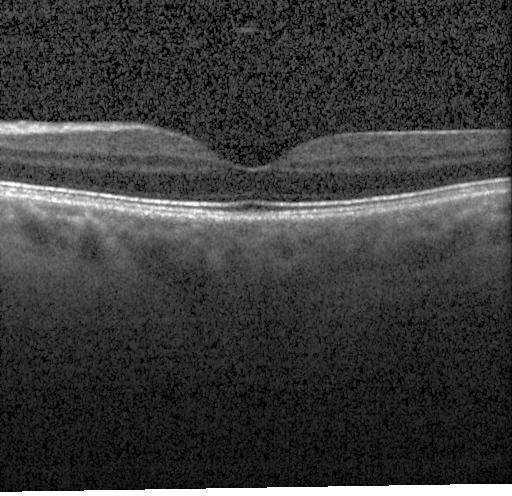 OCT line scan
This B-scan demonstrates no choroidal neovascularization, no diabetic macular edema, and no drusen.